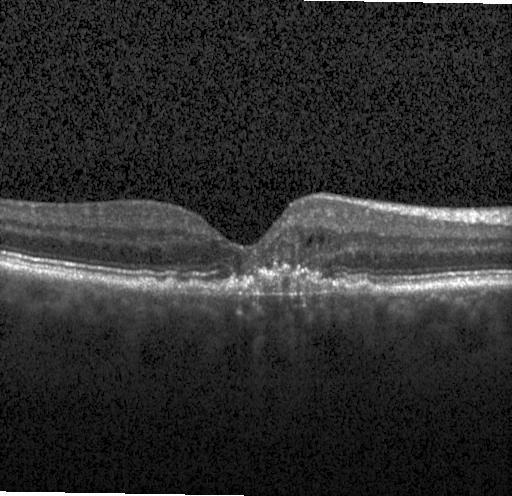

Retinal OCT B-scan.
Diagnosis: CNV.